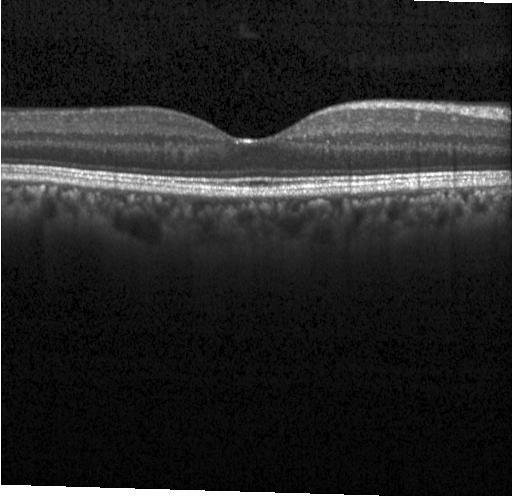 Macular OCT: no evidence of choroidal neovascularization, diabetic macular edema, or drusen.